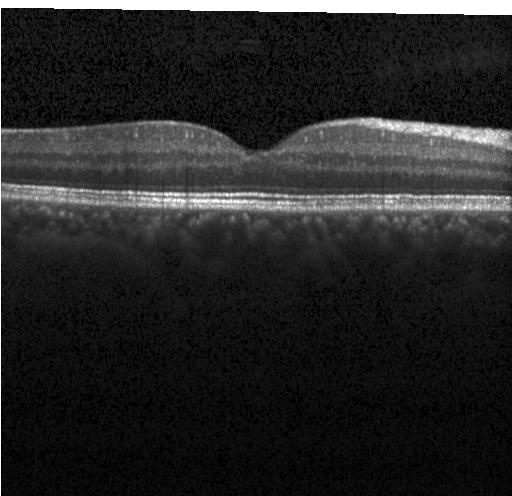

Optical coherence tomography scan, instrument: Heidelberg Spectralis, spectral-domain OCT — Diagnosis: neither choroidal neovascularization, diabetic macular edema, nor drusen.